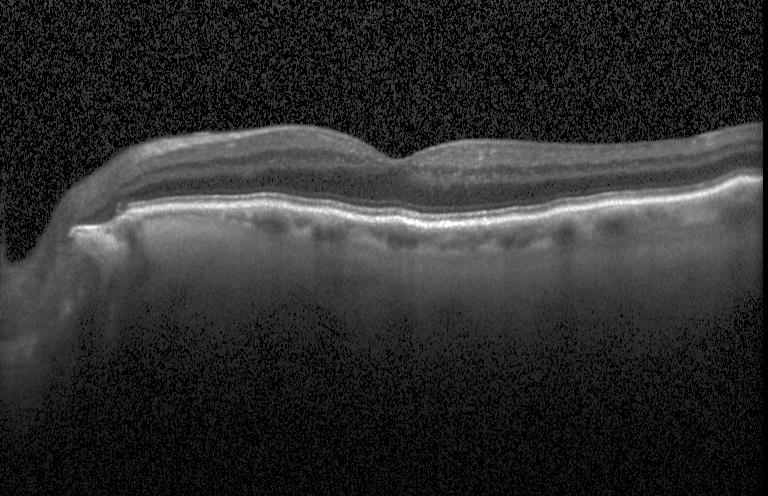
Optical coherence tomography scan
No evidence of choroidal neovascularization, diabetic macular edema, or drusen.